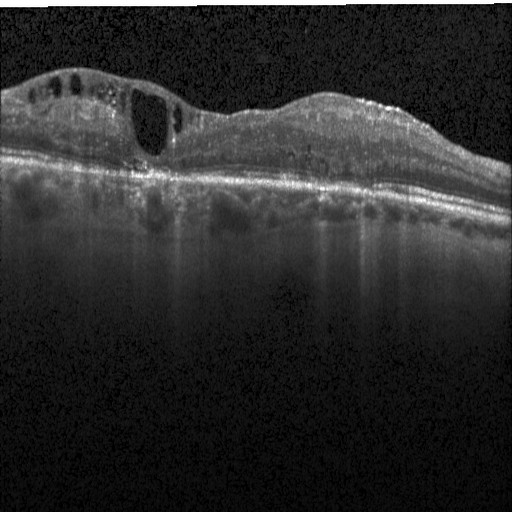 Optical coherence tomography scan; spectral-domain OCT; instrument: Heidelberg Spectralis — Macular OCT: diabetic macular edema (DME).